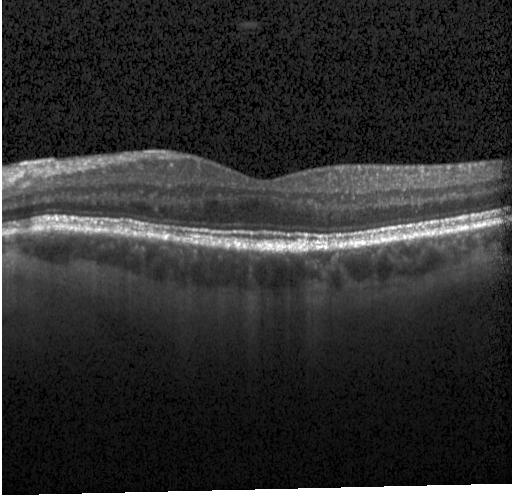 Through the macula; OCT B-scan; instrument: Heidelberg Spectralis. The scan shows no choroidal neovascularization, diabetic macular edema, or drusen.